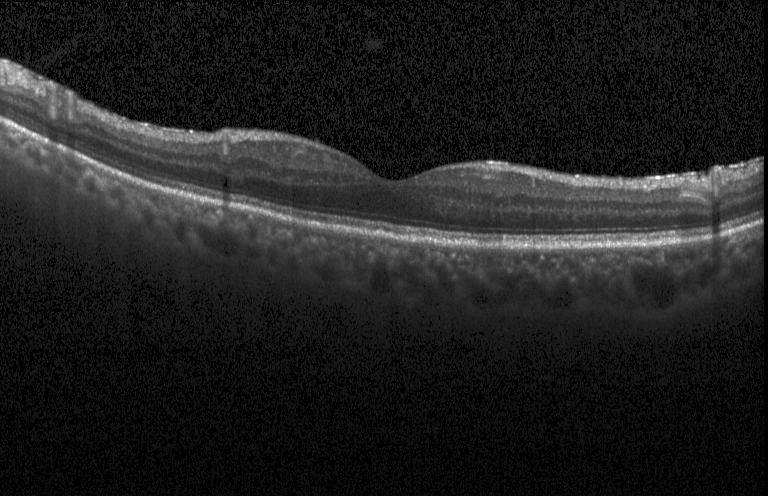
OCT scan showing neither CNV, DME, nor drusen.